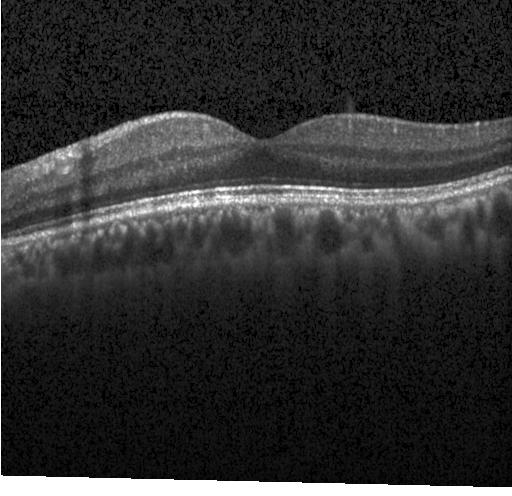
Retinal OCT B-scan — Finding: no choroidal neovascularization, no diabetic macular edema, and no drusen.